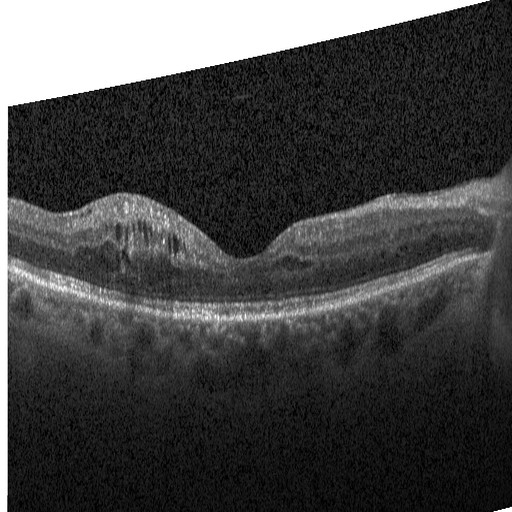 Optical coherence tomography scan. The scan shows DME.